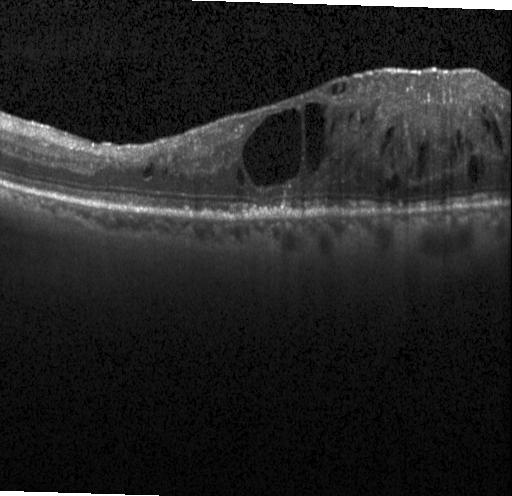

OCT B-scan. Spectral-domain optical coherence tomography. Instrument: Heidelberg Spectralis. OCT finding: DME.